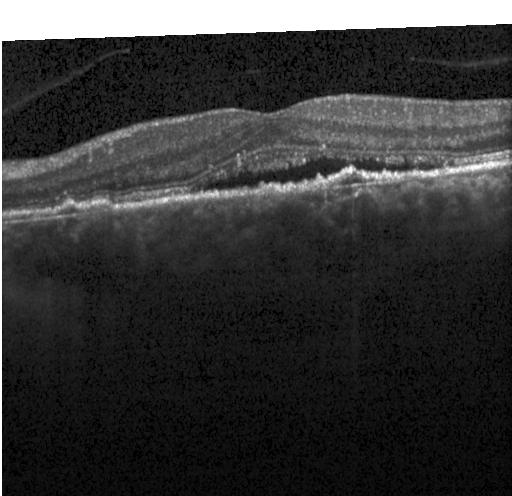
Macular OCT demonstrating CNV.